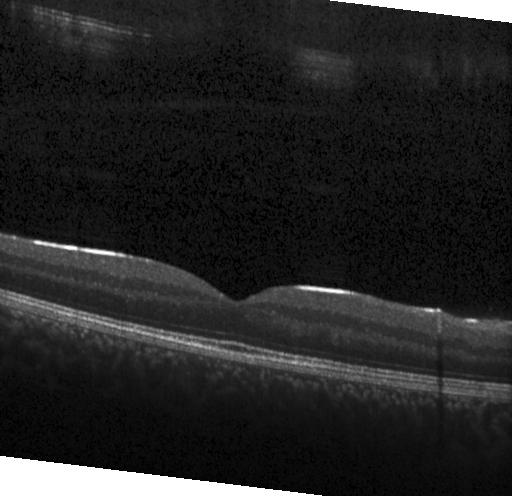

OCT finding: no CNV, no DME, and no drusen.